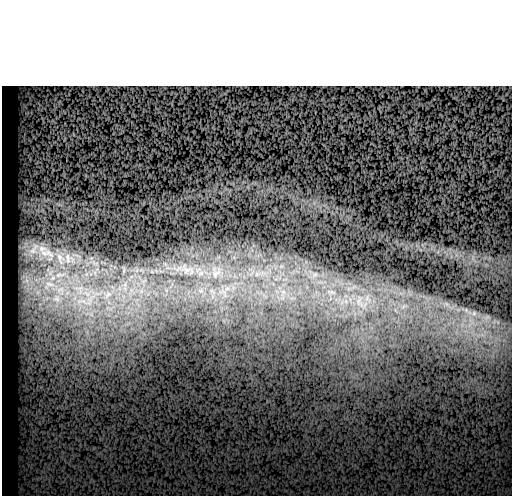

Acquired on a Heidelberg Spectralis · optical coherence tomography B-scan · spectral-domain OCT — This B-scan demonstrates a choroidal neovascular membrane.